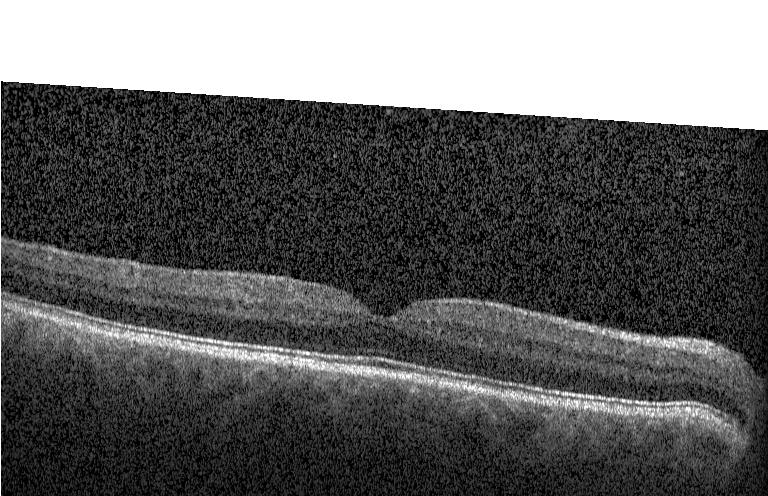

Instrument: Heidelberg Spectralis. Spectral-domain optical coherence tomography. Optical coherence tomography scan. Through the macula
No evidence of CNV, DME, or drusen.